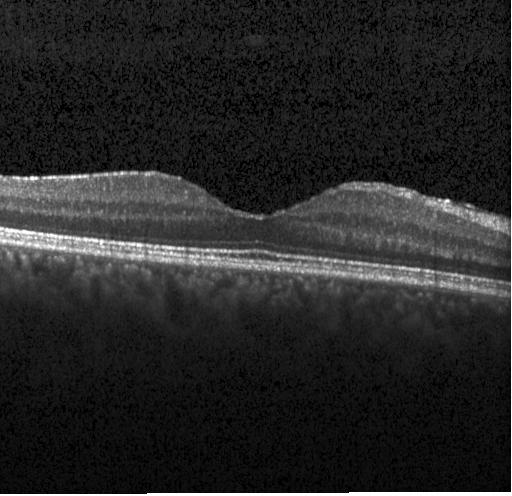

Dx: no choroidal neovascularization, diabetic macular edema, or drusen.